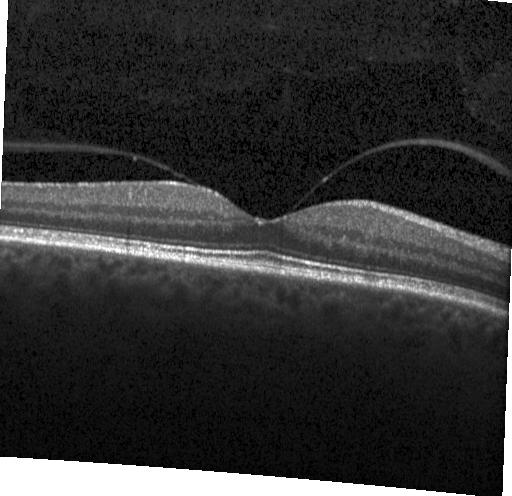 Fovea-centered, SD-OCT, optical coherence tomography B-scan, Heidelberg Spectralis OCT system
Diagnosis: no evidence of CNV, DME, or drusen.